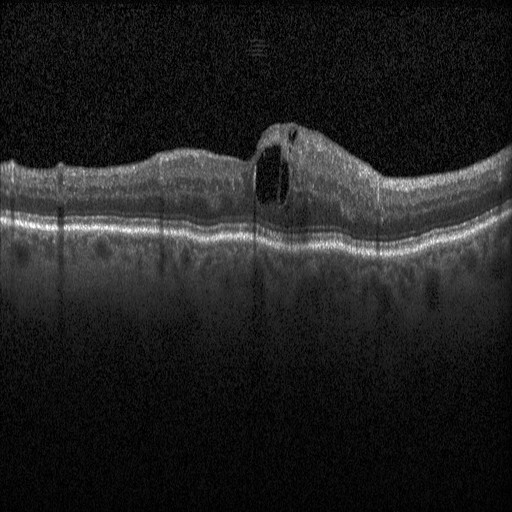 Spectral-domain OCT B-scan: DME.